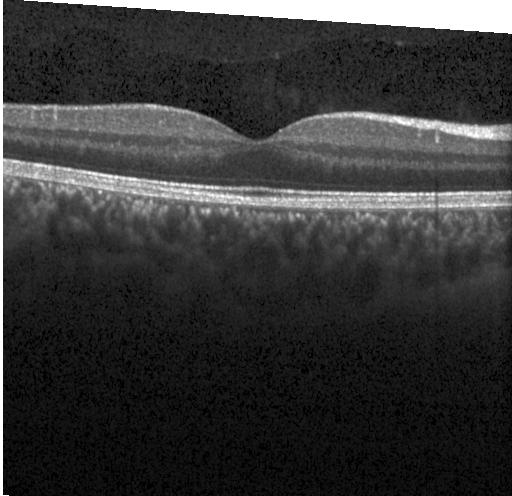

Spectral-domain OCT, fovea-centered, retinal OCT B-scan, instrument: Heidelberg Spectralis.
Finding: neither choroidal neovascularization, diabetic macular edema, nor drusen.